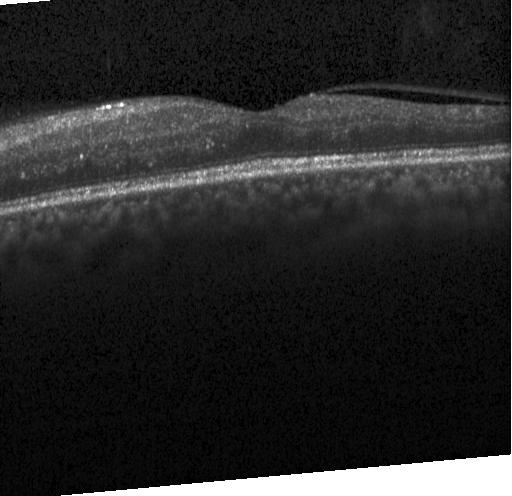 Diagnosis: diabetic macular edema (DME).